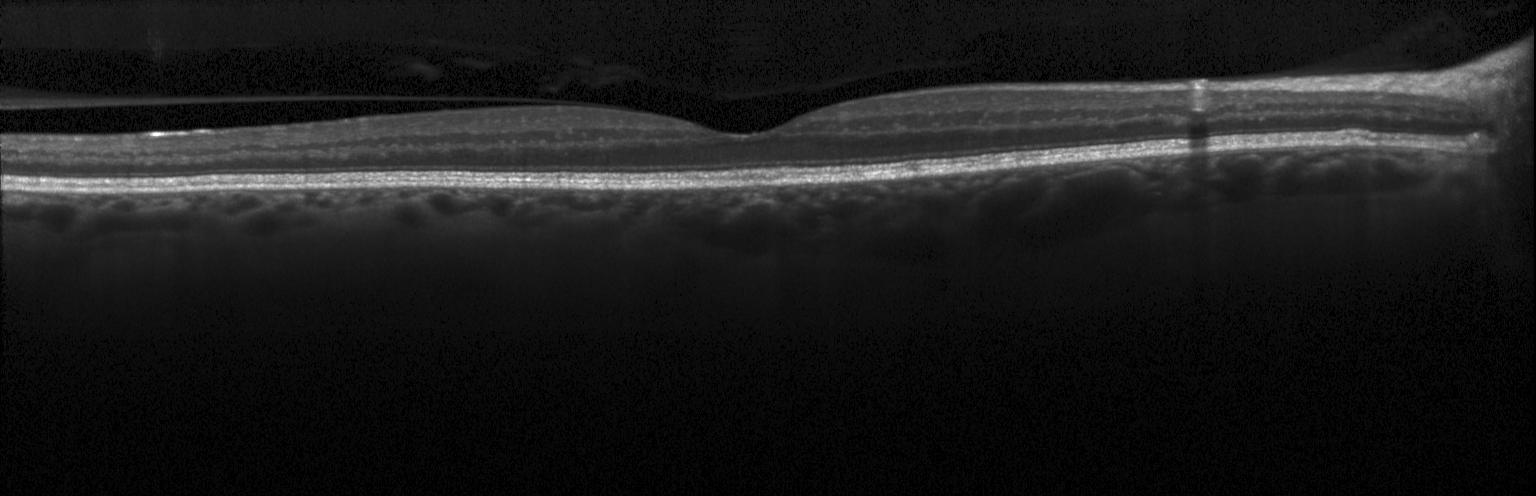
Diagnosis: no evidence of CNV, DME, or drusen.